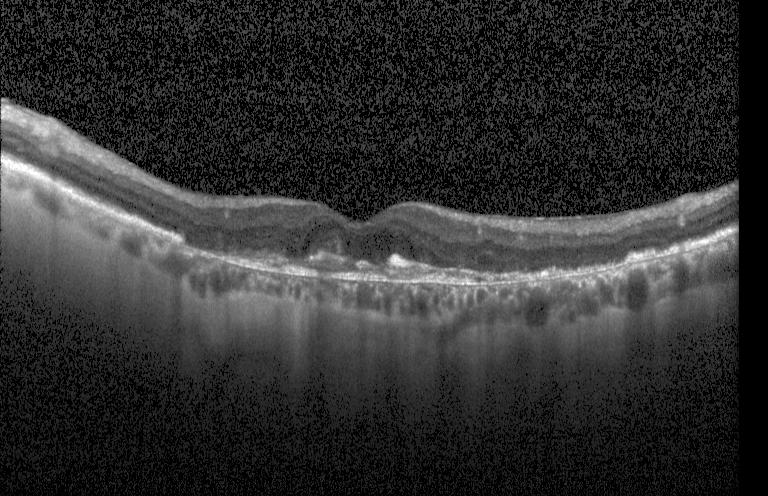 Heidelberg Spectralis. Optical coherence tomography B-scan. Spectral-domain optical coherence tomography.
Impression: a choroidal neovascular membrane.